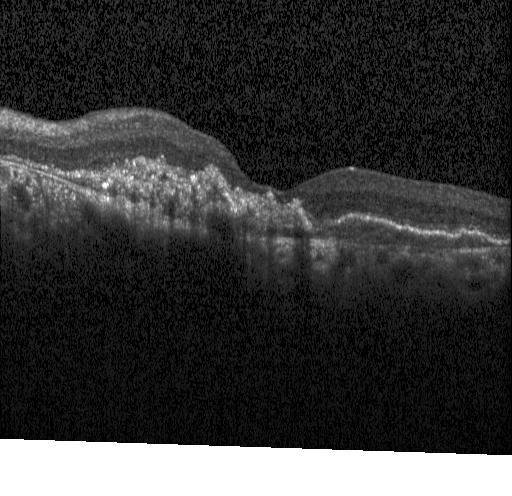
Retinal OCT cross-section
Impression: a choroidal neovascular membrane.